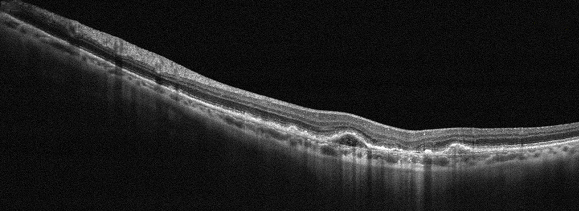

OCT B-scan, oculus sinister. Impression: AMD.